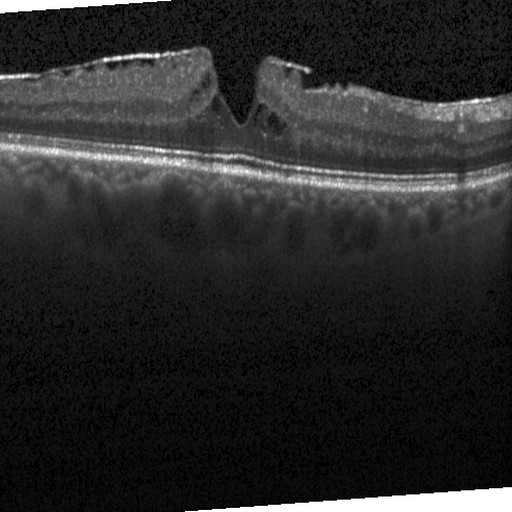
Dx: diabetic macular edema (DME).